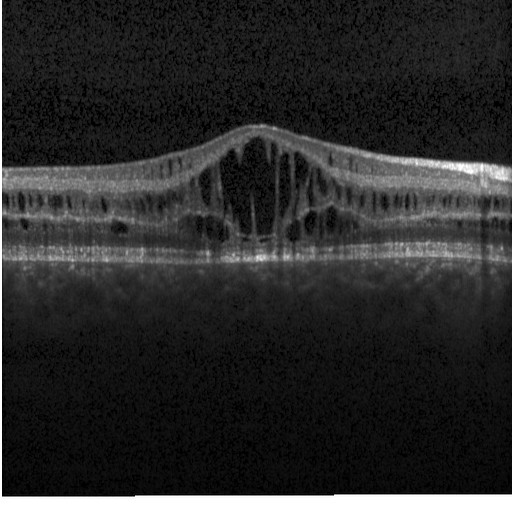
Retinal OCT cross-section. Finding: diabetic macular edema (DME).